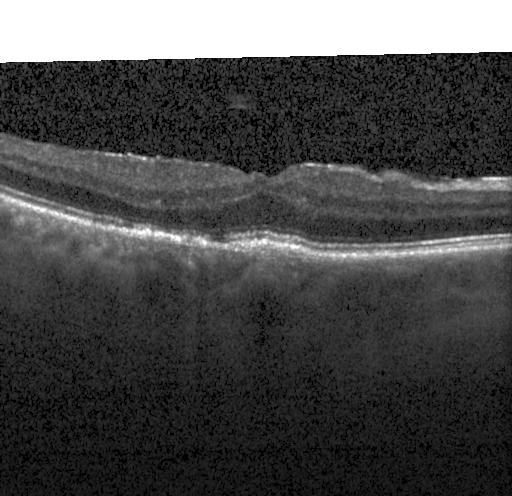

Spectral-domain OCT; OCT line scan; centered on the fovea; instrument: Heidelberg Spectralis. OCT finding: choroidal neovascularization.